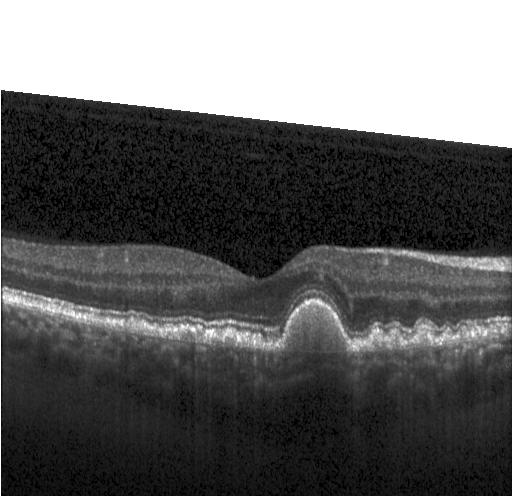

Finding: sub-RPE drusenoid deposits.